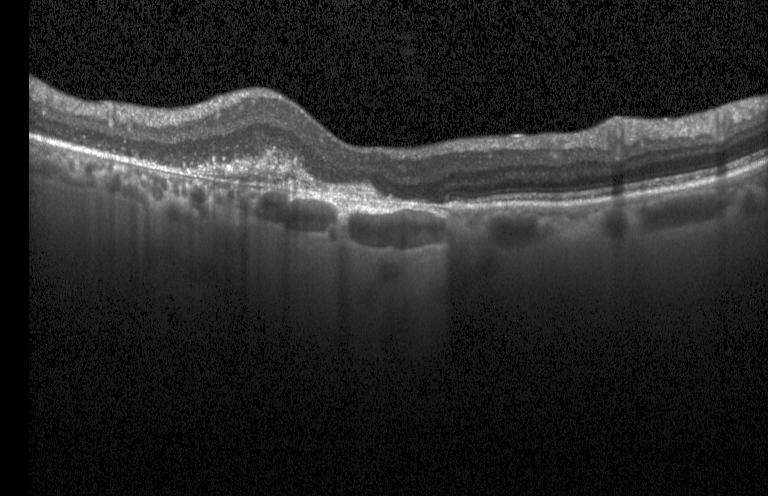 Retinal OCT B-scan. Fovea-centered. Acquired on a Heidelberg Spectralis — Choroidal neovascularization (CNV).